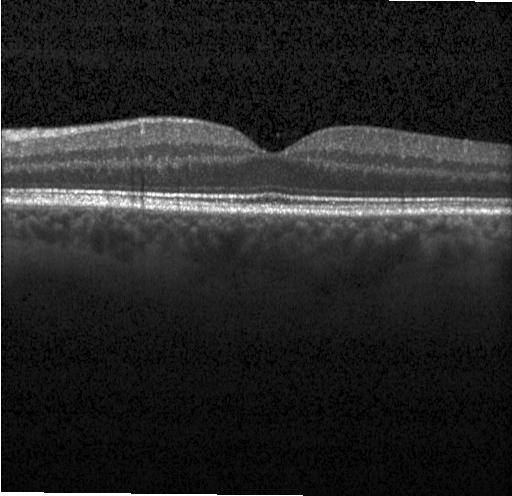
Impression: neither CNV, DME, nor drusen.